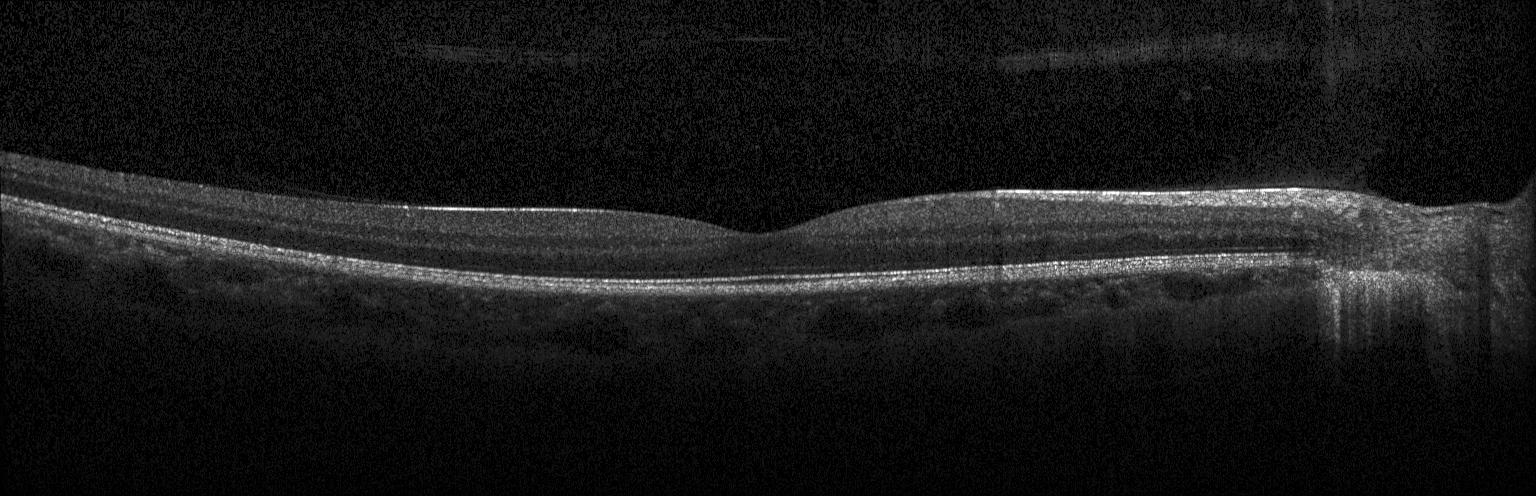
Diagnosis: no choroidal neovascularization, no diabetic macular edema, and no drusen.